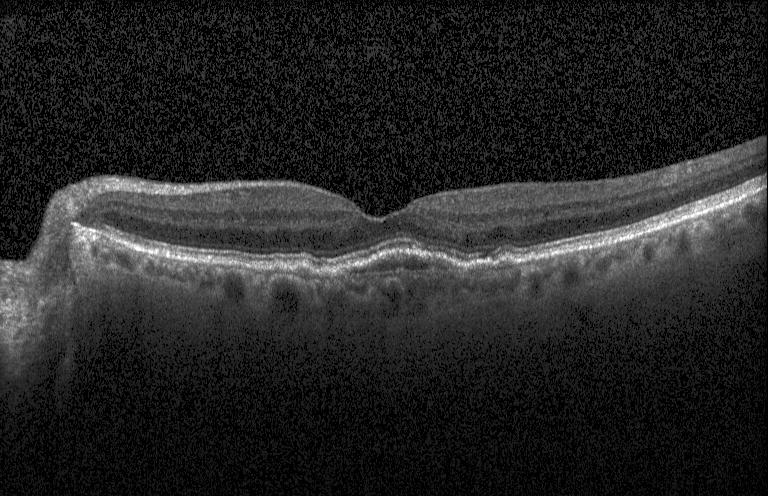
Diagnosis: choroidal neovascularization (CNV).